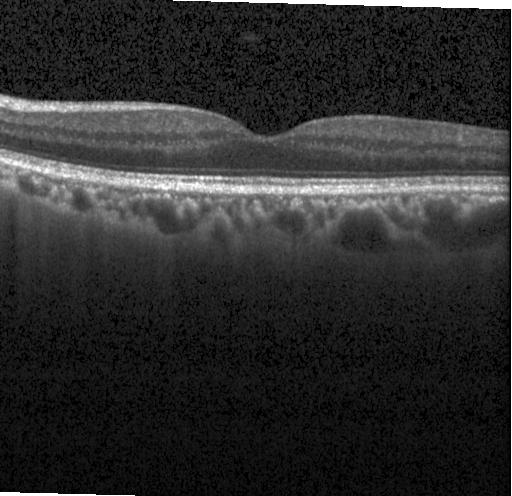
No CNV, DME, or drusen.